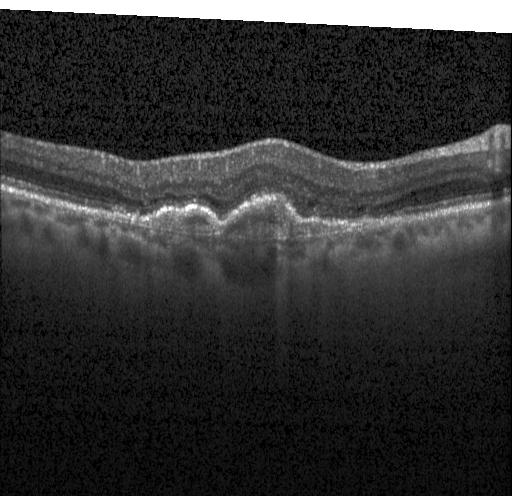

OCT B-scan showing CNV.